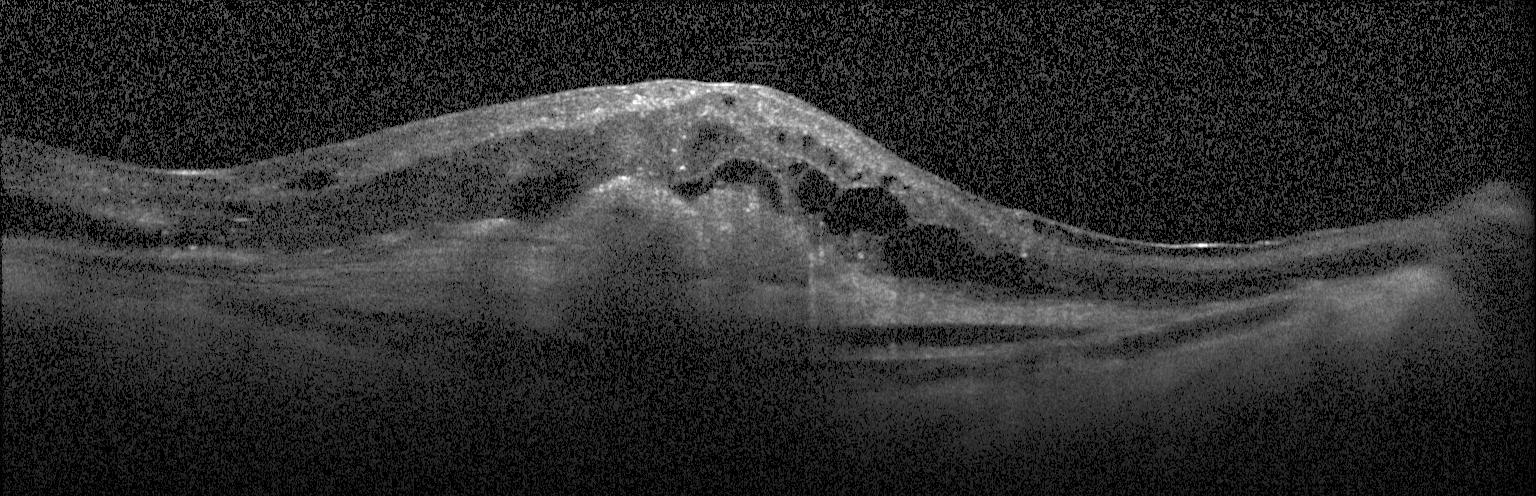

Centered on the fovea, retinal OCT cross-section, Heidelberg Spectralis, spectral-domain optical coherence tomography.
The scan shows choroidal neovascularization (CNV).